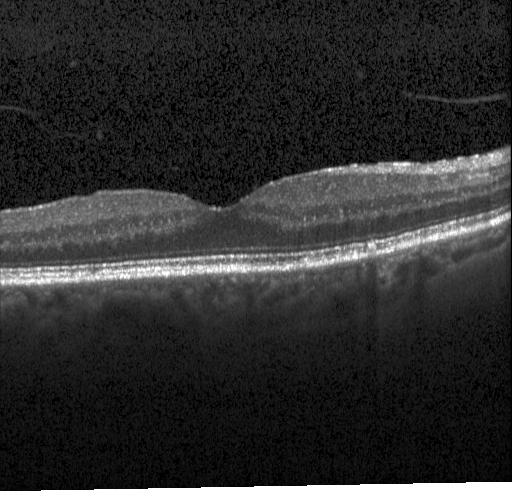

Finding: neither choroidal neovascularization, diabetic macular edema, nor drusen.